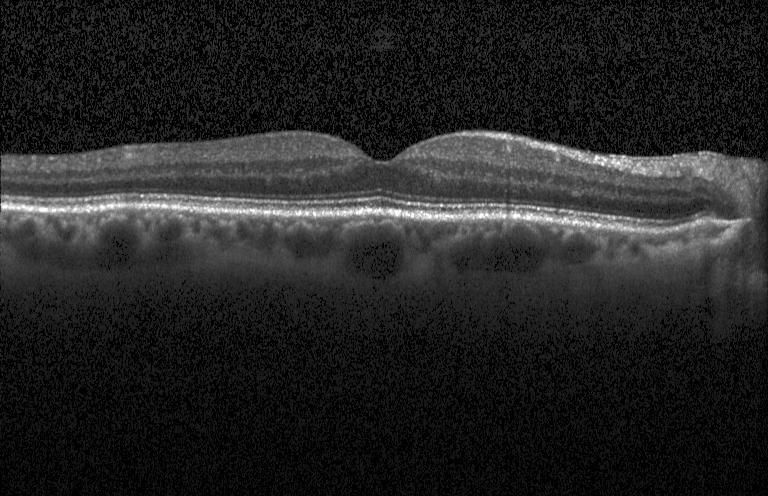

Heidelberg Spectralis OCT system; retinal OCT cross-section; centered on the fovea. Impression: no choroidal neovascularization, no diabetic macular edema, and no drusen.